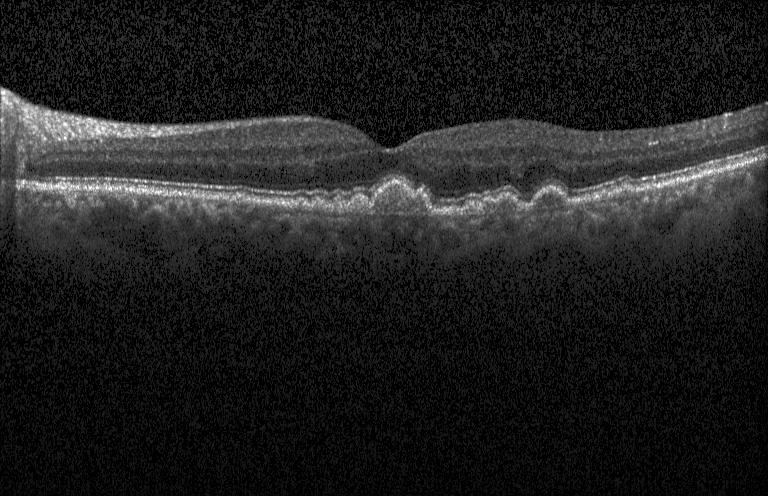

Heidelberg Spectralis OCT system · macular scan · OCT line scan. The scan shows sub-RPE drusenoid deposits.